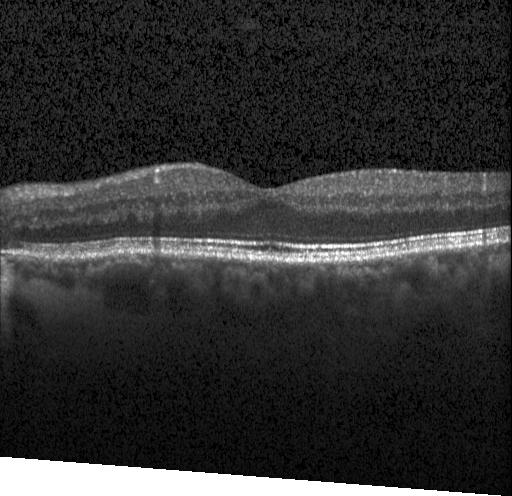 Spectral-domain optical coherence tomography, retinal OCT B-scan. The scan shows no CNV, no DME, and no drusen.